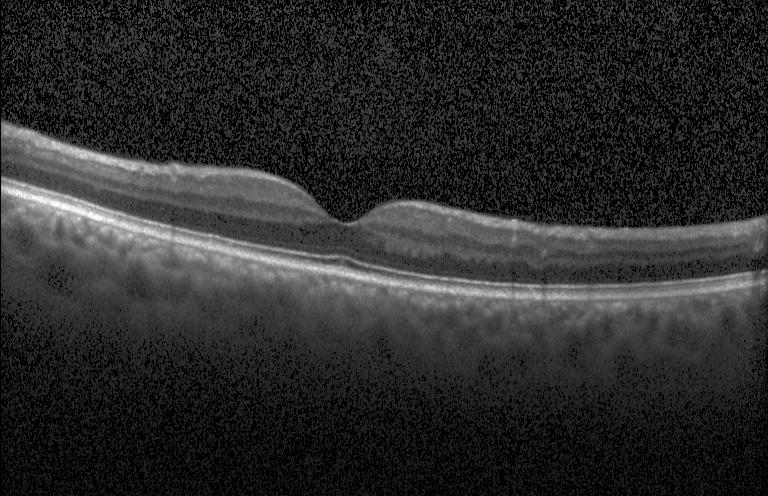
OCT B-scan, instrument: Heidelberg Spectralis, through the macula — Dx: no CNV, DME, or drusen.